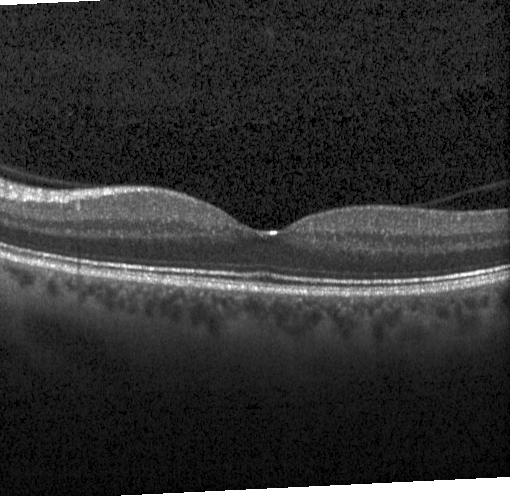
Optical coherence tomography B-scan. Spectral-domain optical coherence tomography. Horizontal scan through the fovea. Acquired on a Heidelberg Spectralis. The scan shows no choroidal neovascularization, diabetic macular edema, or drusen.